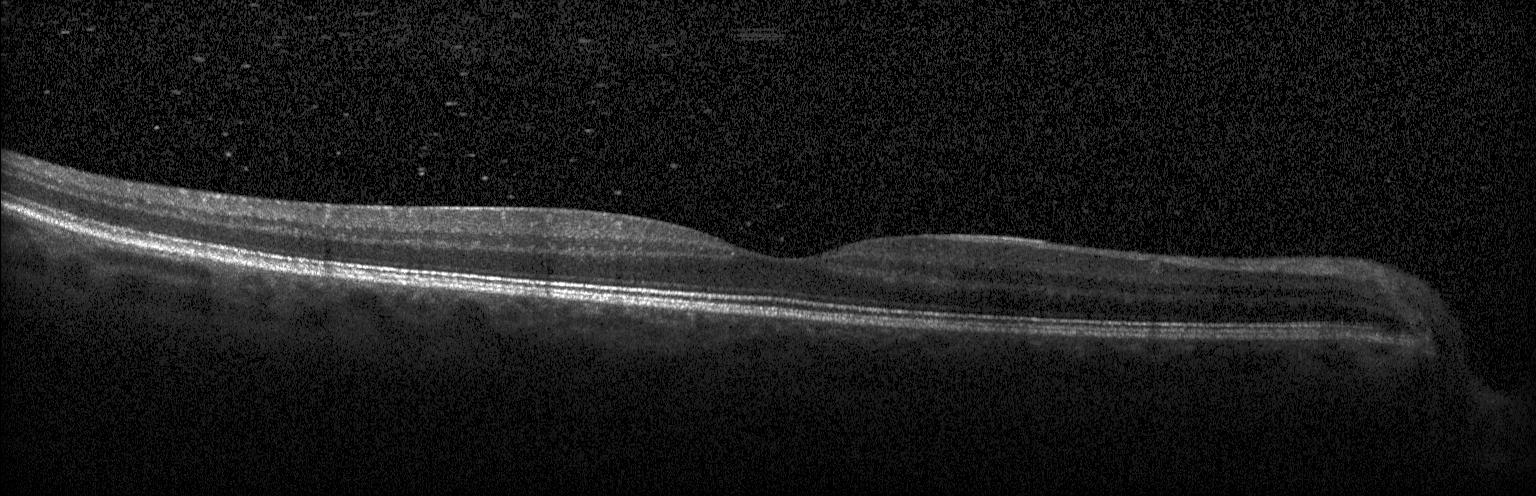
Retinal OCT cross-section showing neither choroidal neovascularization, diabetic macular edema, nor drusen.